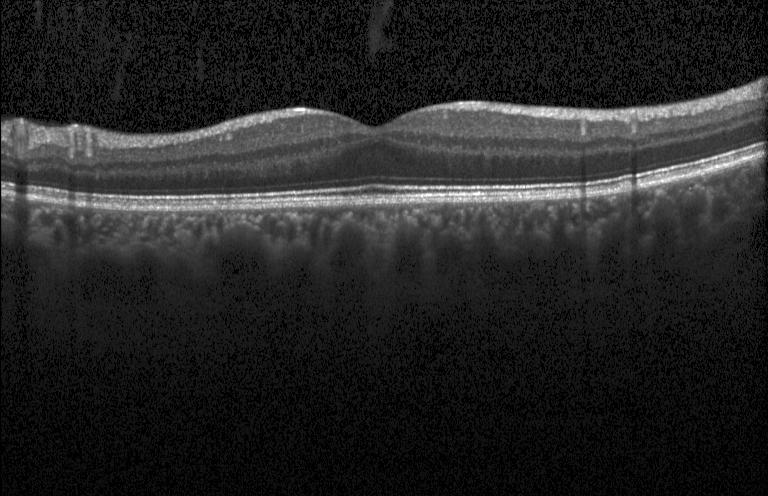

Spectral-domain OCT B-scan: no evidence of choroidal neovascularization, diabetic macular edema, or drusen.